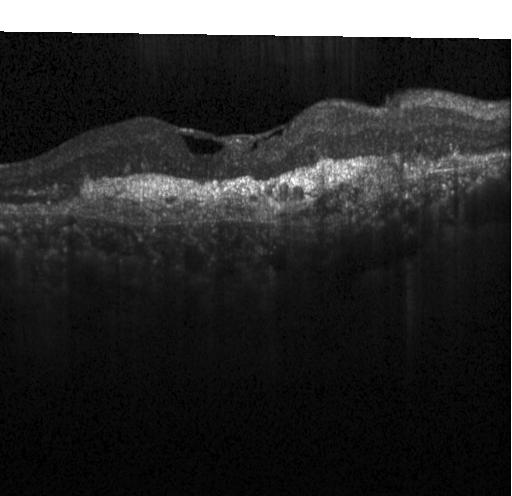
Spectral-domain OCT, optical coherence tomography scan, through the macula — Impression: choroidal neovascularization (CNV).